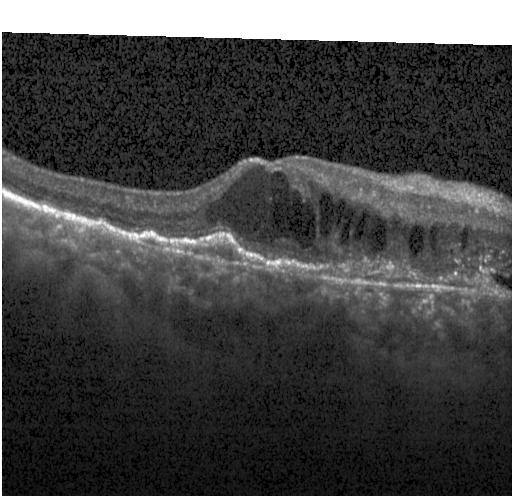

The scan shows choroidal neovascularization (CNV).